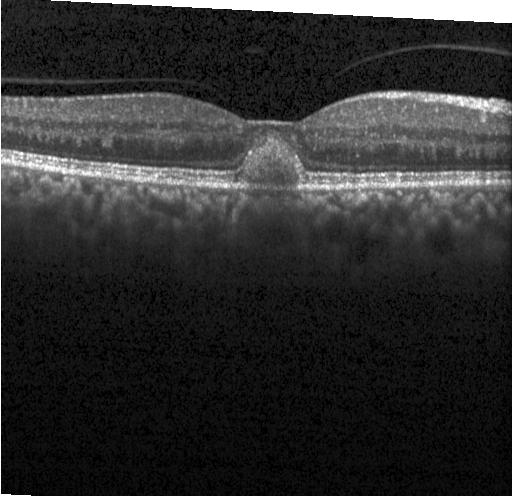 Fovea-centered. Instrument: Heidelberg Spectralis. Spectral-domain OCT. Retinal OCT B-scan.
OCT finding: a choroidal neovascular membrane.